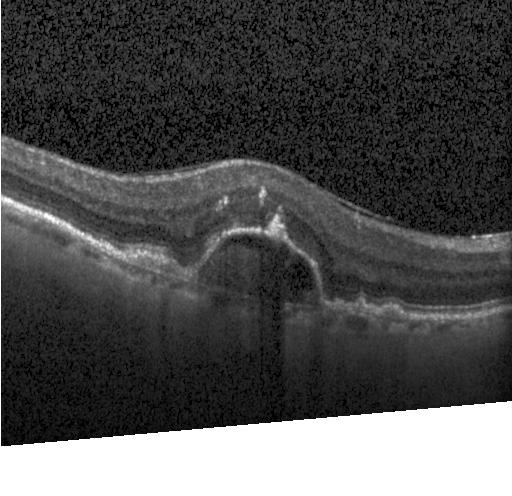

Macular OCT: a choroidal neovascular membrane.